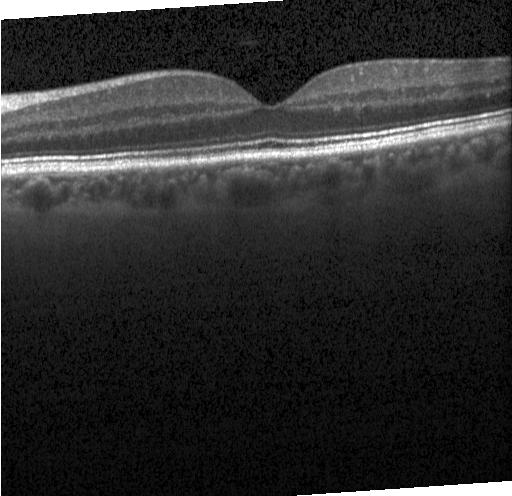

Fovea-centered, retinal OCT B-scan — Impression: no CNV, no DME, and no drusen.